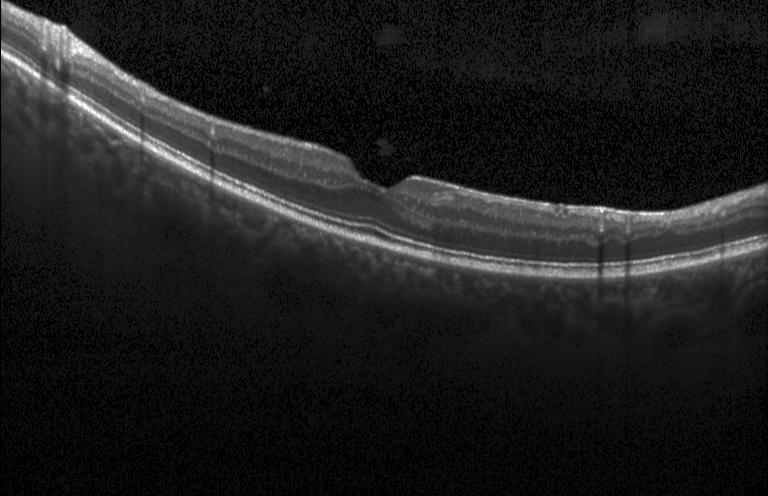

OCT B-scan showing neither CNV, DME, nor drusen.